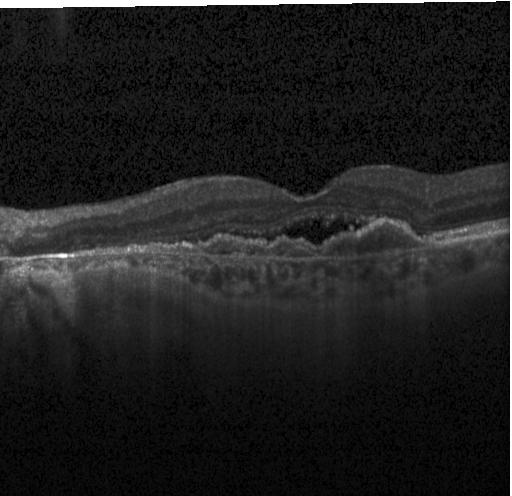 The scan shows CNV.